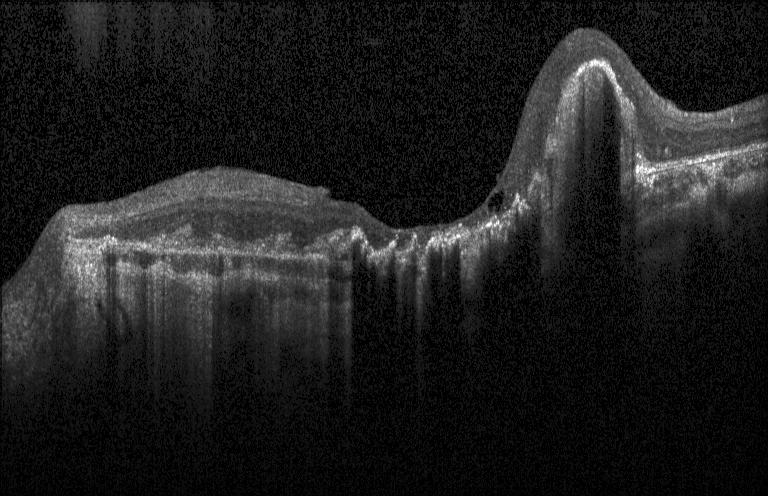 Retinal OCT B-scan — Diagnosis: choroidal neovascularization (CNV).